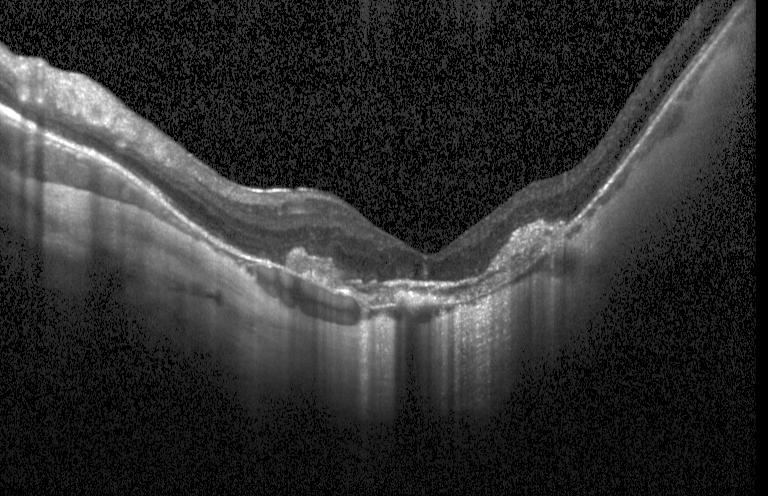
Impression: a choroidal neovascular membrane.